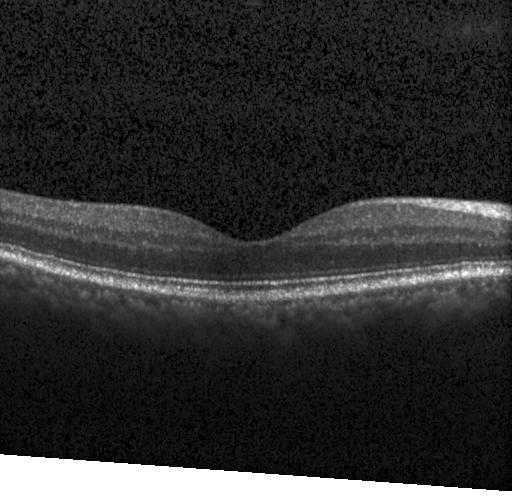 Finding: neither CNV, DME, nor drusen.